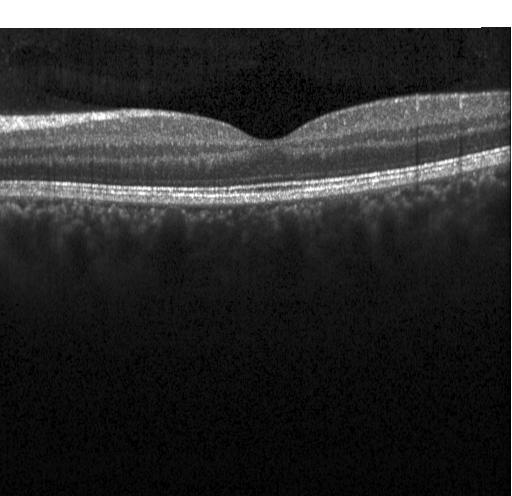

Macular OCT demonstrating no evidence of choroidal neovascularization, diabetic macular edema, or drusen.